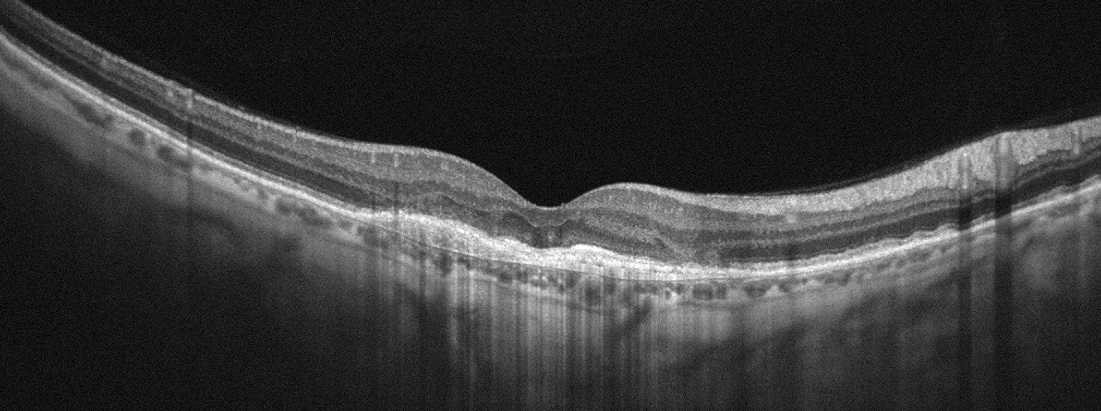 Fovea-centered. Retinal OCT B-scan. Optovue Avanti RTVue XR
Age-related macular degeneration.